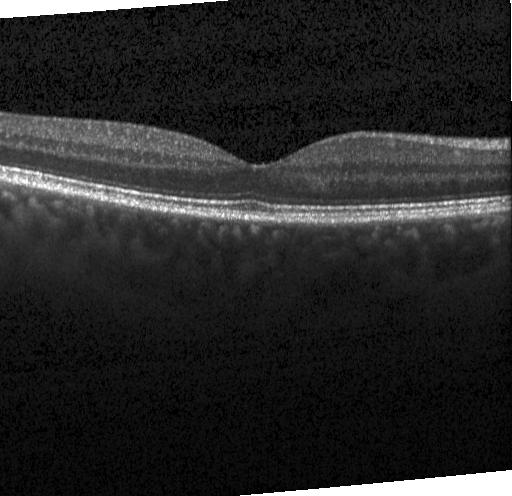 Optical coherence tomography scan · spectral-domain optical coherence tomography. No evidence of CNV, DME, or drusen.